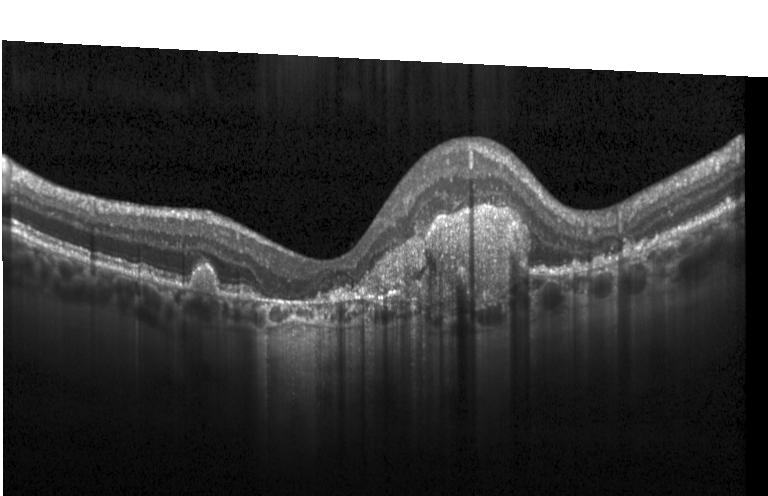

Heidelberg Spectralis OCT system, through the macula, optical coherence tomography B-scan, spectral-domain OCT.
This B-scan demonstrates a choroidal neovascular membrane.